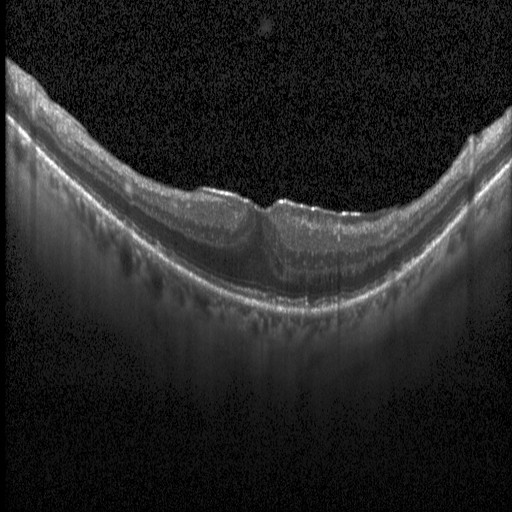 Spectral-domain OCT B-scan: DME.